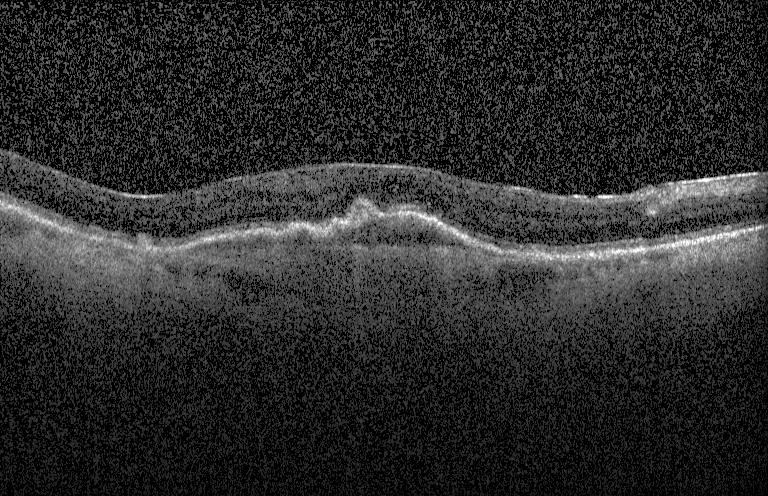

Spectral-domain optical coherence tomography, OCT B-scan. Macular OCT: a choroidal neovascular membrane.